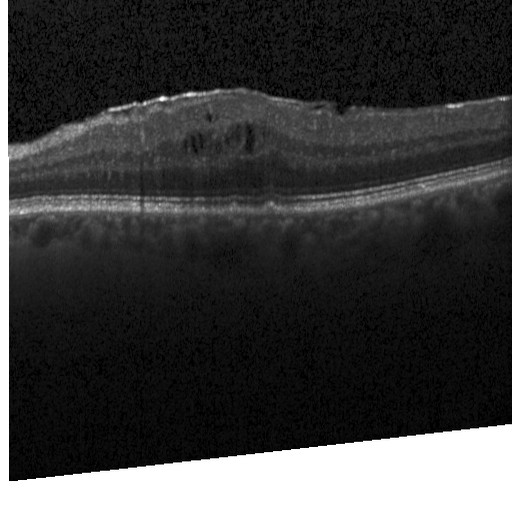
SD-OCT. Retinal OCT B-scan. Heidelberg Spectralis OCT system — Impression: diabetic macular edema (DME).